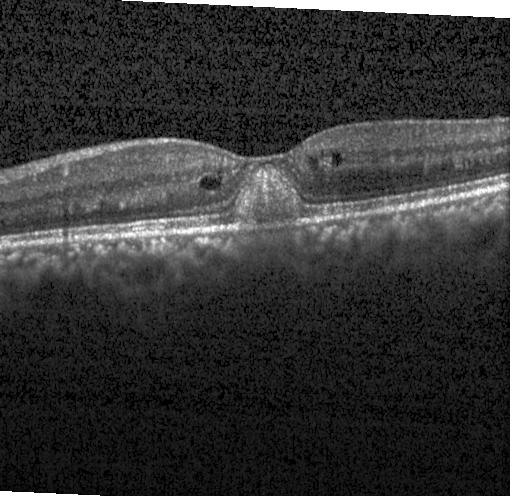

Macular scan, instrument: Heidelberg Spectralis, SD-OCT, retinal OCT cross-section
Finding: CNV.